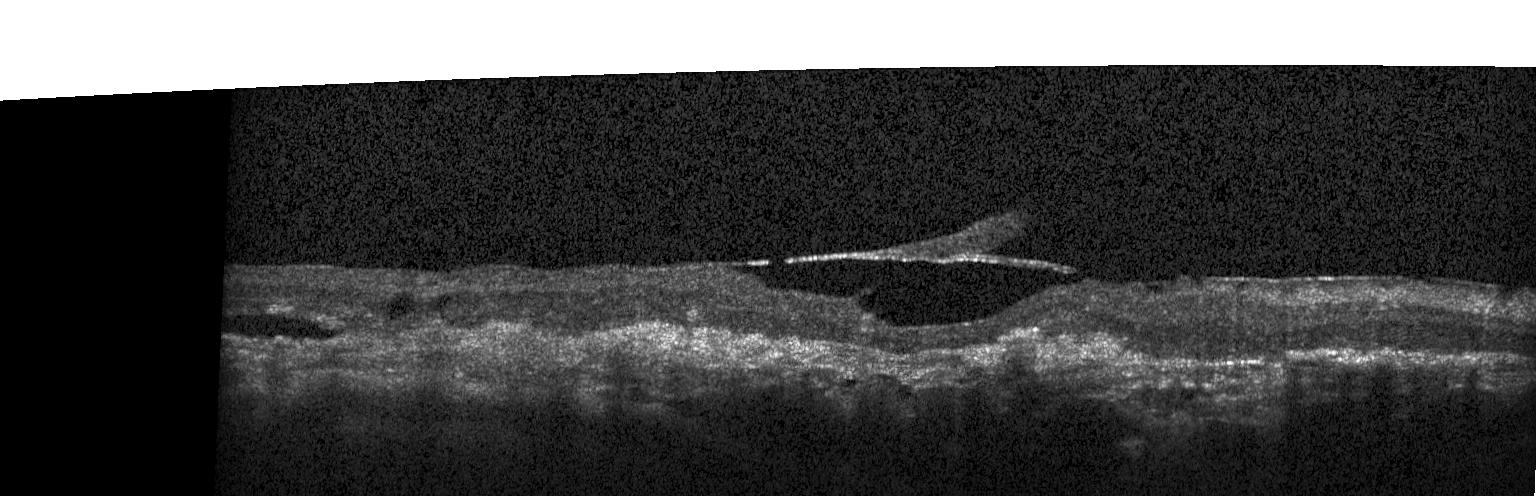
Spectral-domain optical coherence tomography, through the macula, Heidelberg Spectralis, OCT B-scan
Dx: a choroidal neovascular membrane.